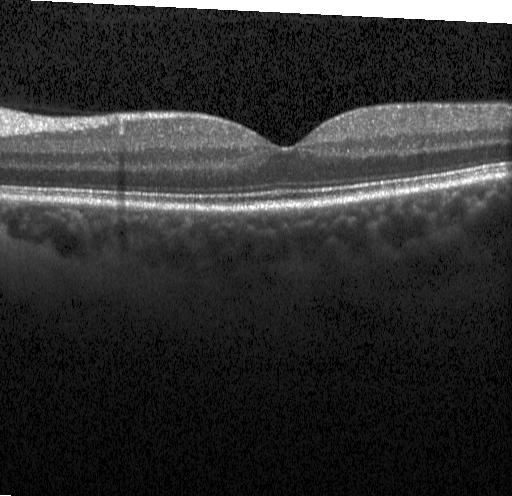

Retinal OCT cross-section, acquired on a Heidelberg Spectralis, spectral-domain optical coherence tomography, through the macula — Diagnosis: neither CNV, DME, nor drusen.